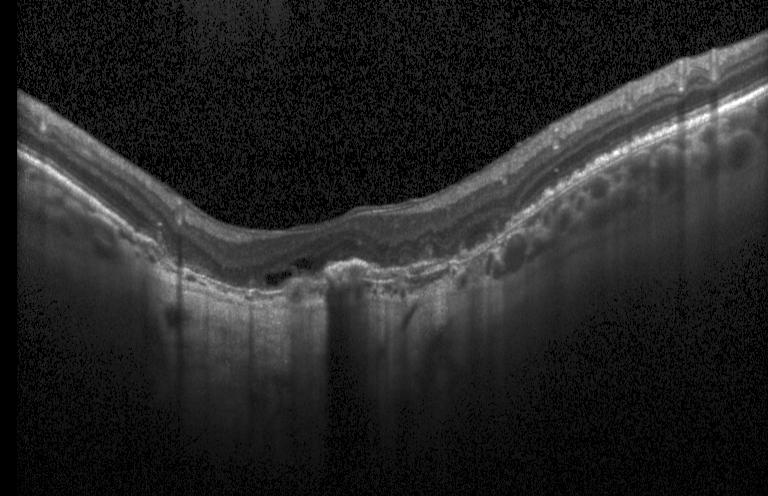

SD-OCT. Retinal OCT cross-section.
OCT finding: choroidal neovascularization (CNV).